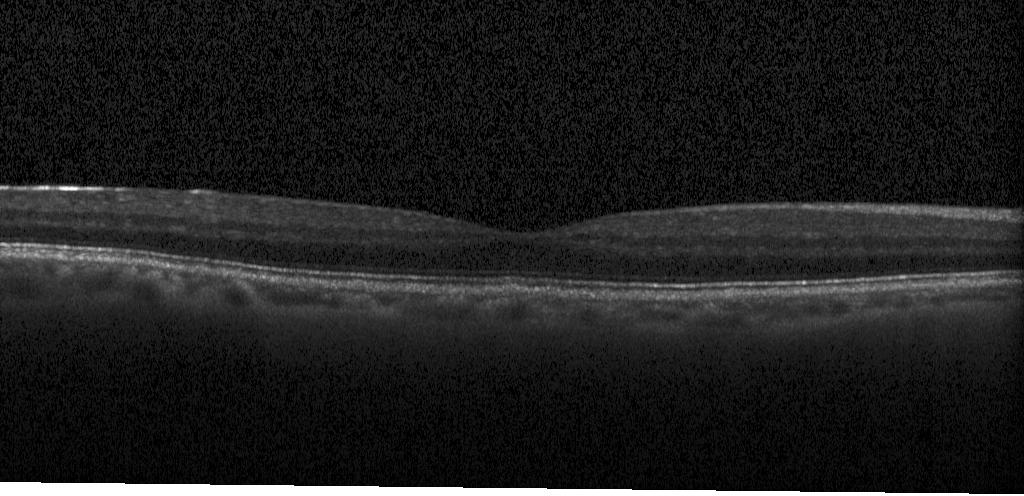
Retinal OCT cross-section. No choroidal neovascularization, no diabetic macular edema, and no drusen.